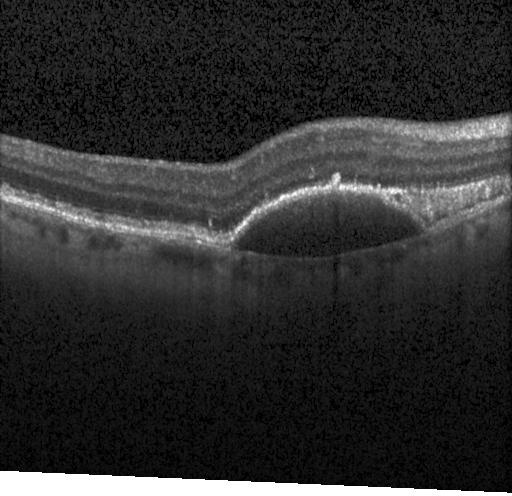
Impression: choroidal neovascularization.